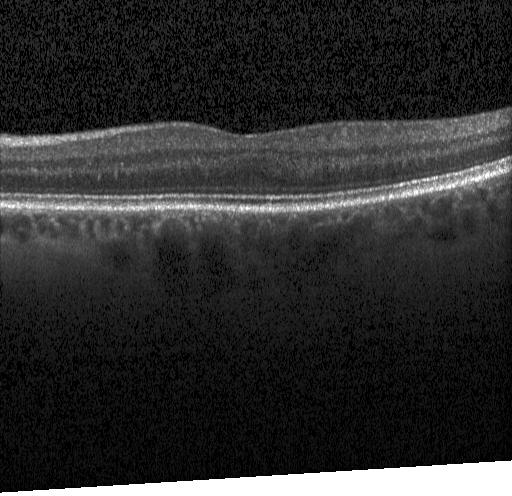

Spectral-domain OCT, optical coherence tomography scan
Impression: neither choroidal neovascularization, diabetic macular edema, nor drusen.